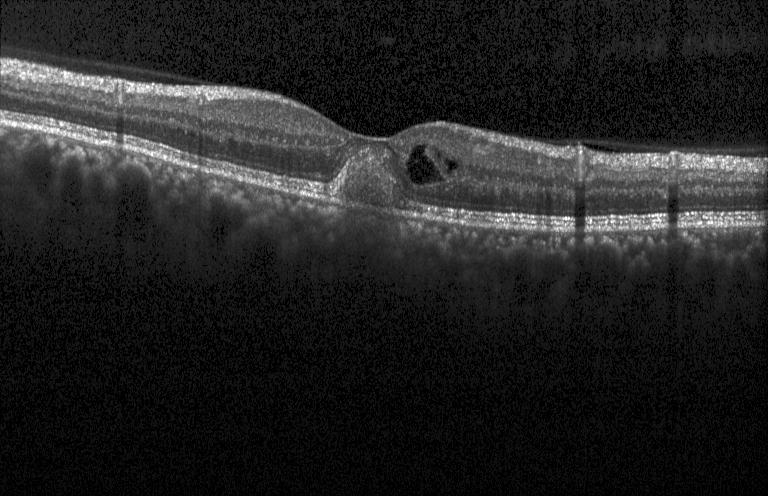 Macular OCT: a choroidal neovascular membrane.